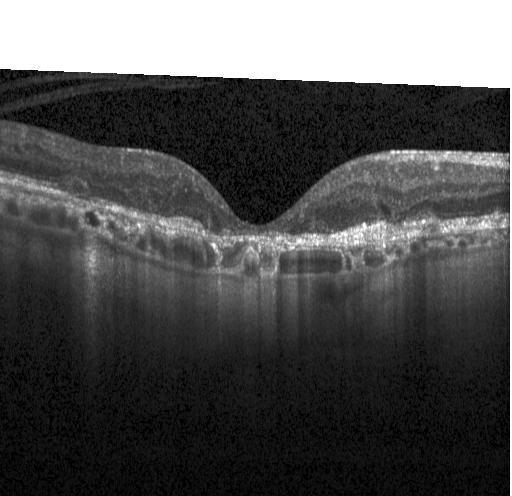
Spectral-domain optical coherence tomography; acquired on a Heidelberg Spectralis; optical coherence tomography B-scan.
Impression: a choroidal neovascular membrane.